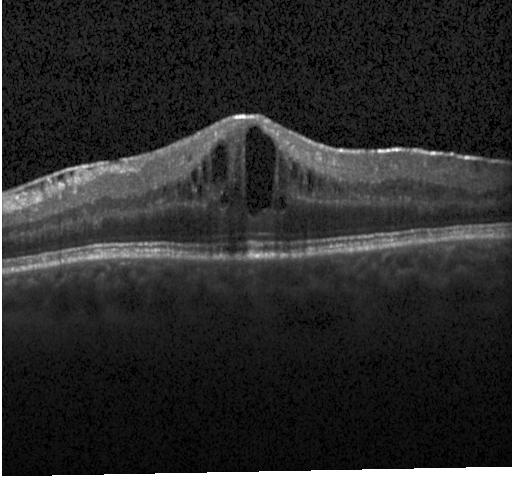

Acquired on a Heidelberg Spectralis, SD-OCT, macular scan, OCT line scan. Dx: diabetic macular edema.